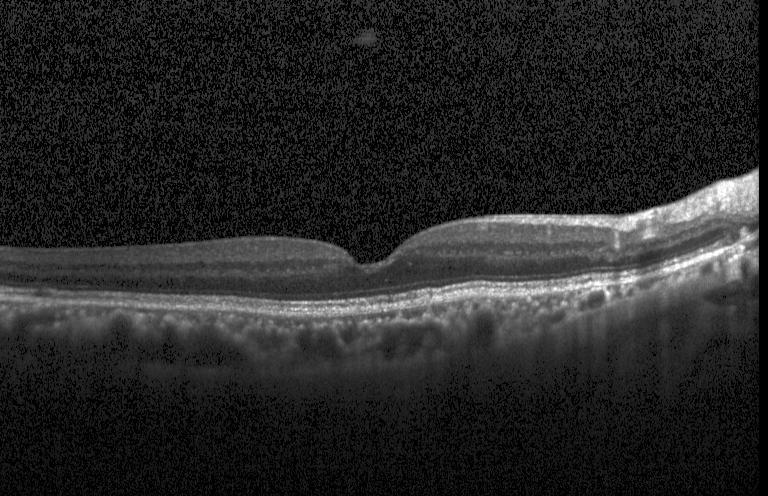
Assessment: neither choroidal neovascularization, diabetic macular edema, nor drusen.